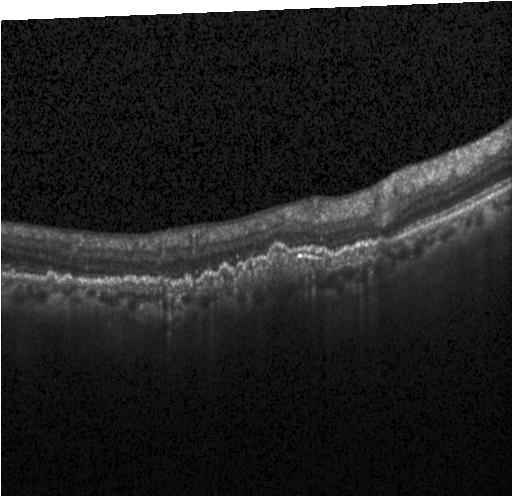

OCT finding: choroidal neovascularization.